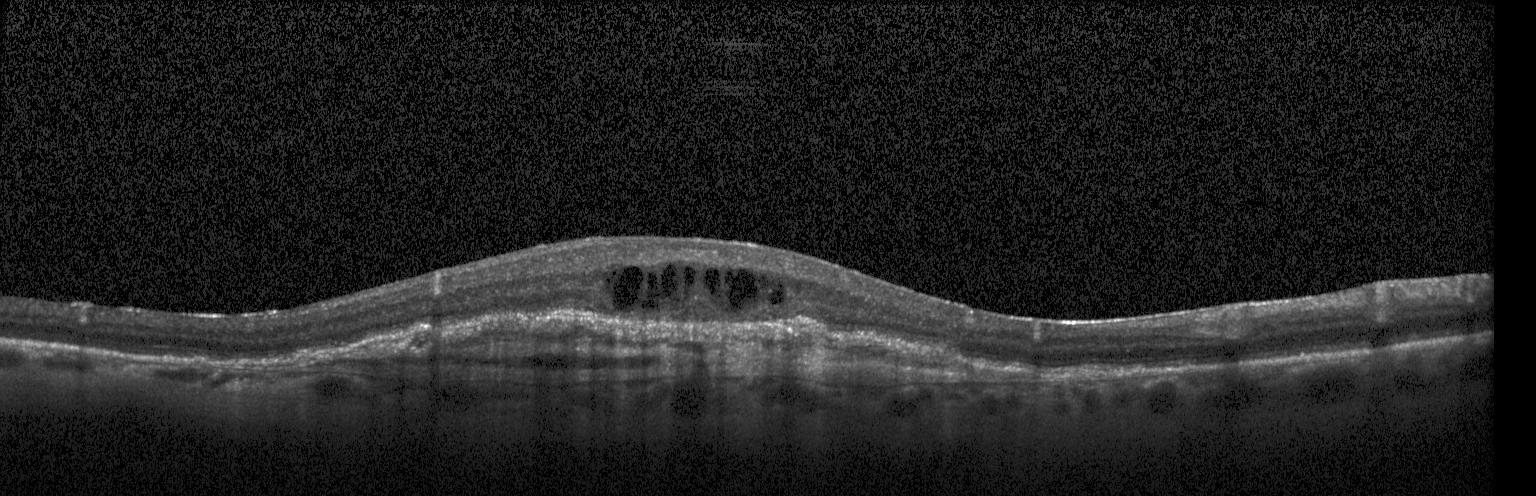 SD-OCT · horizontal scan through the fovea · retinal OCT B-scan · Heidelberg Spectralis. This B-scan demonstrates choroidal neovascularization.